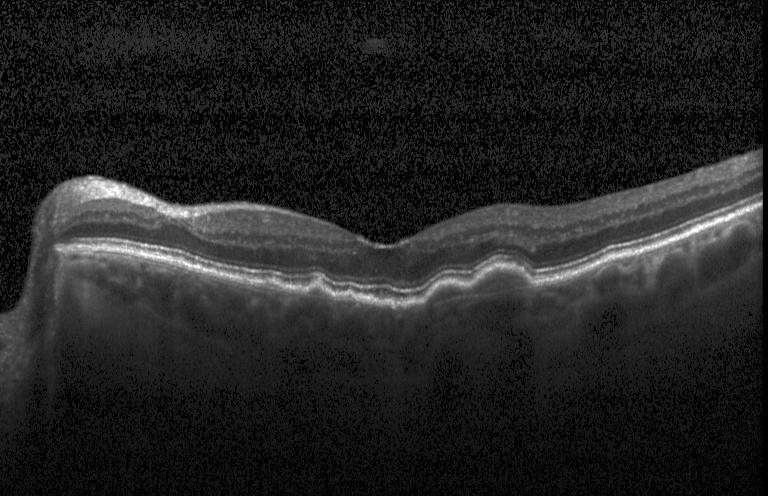 Macular scan, Heidelberg Spectralis OCT system, optical coherence tomography B-scan
Finding: a choroidal neovascular membrane.